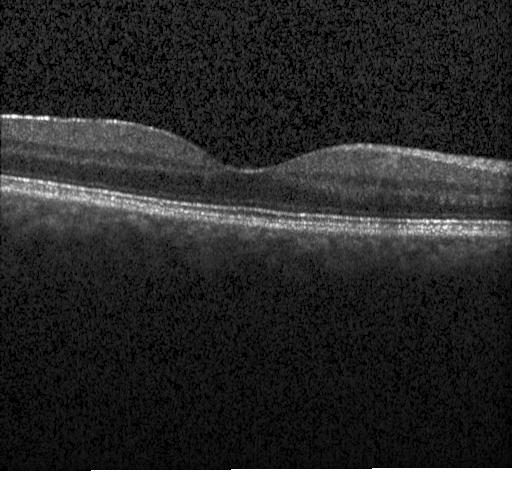 No choroidal neovascularization, diabetic macular edema, or drusen.